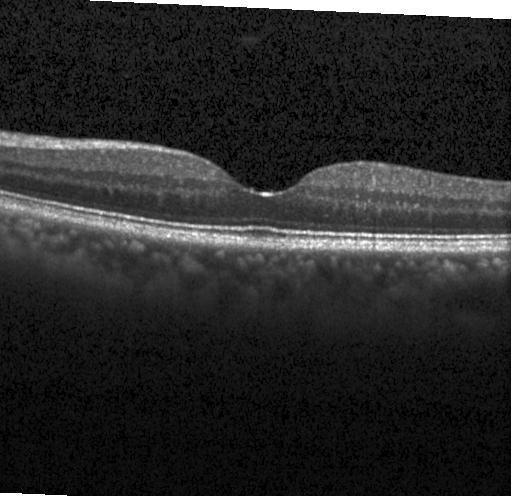

Horizontal scan through the fovea. Optical coherence tomography B-scan. The scan shows no evidence of choroidal neovascularization, diabetic macular edema, or drusen.